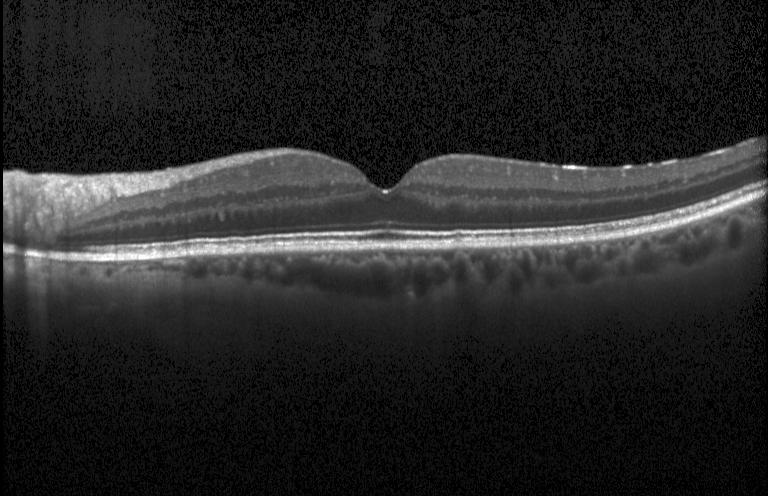 SD-OCT; optical coherence tomography B-scan; instrument: Heidelberg Spectralis — This B-scan demonstrates no evidence of choroidal neovascularization, diabetic macular edema, or drusen.